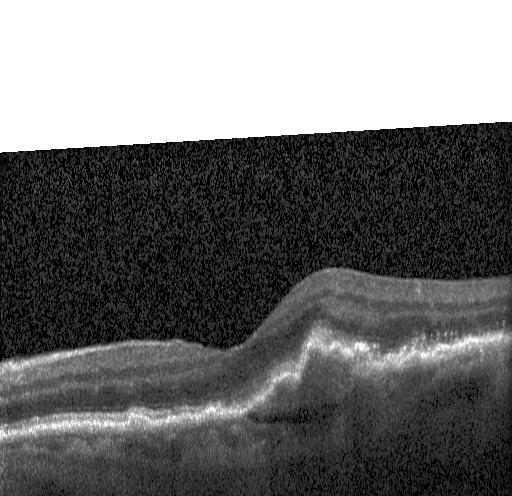 SD-OCT; OCT B-scan; Heidelberg Spectralis. The scan shows a choroidal neovascular membrane.